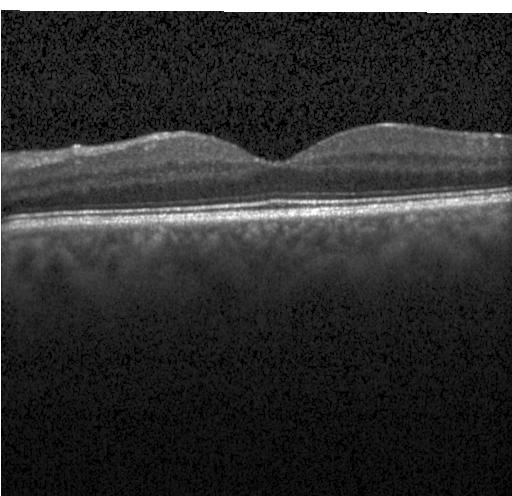
Retinal OCT cross-section · Heidelberg Spectralis · spectral-domain optical coherence tomography · centered on the fovea.
Impression: no evidence of choroidal neovascularization, diabetic macular edema, or drusen.